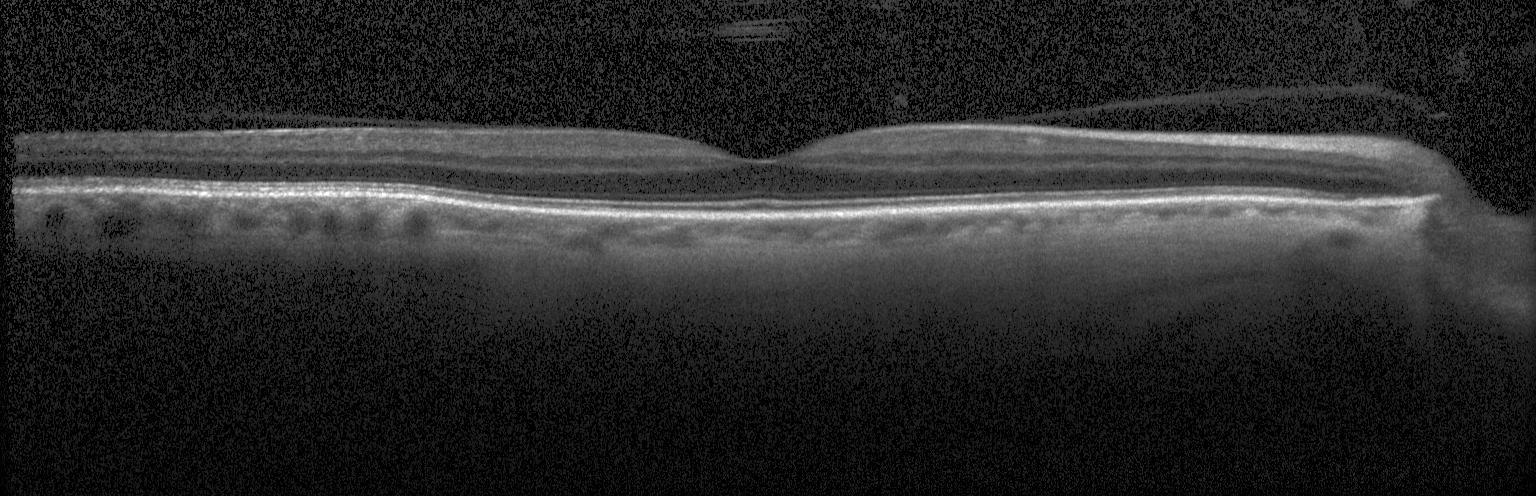 OCT B-scan, through the macula, instrument: Heidelberg Spectralis.
Macular OCT: no choroidal neovascularization, diabetic macular edema, or drusen.